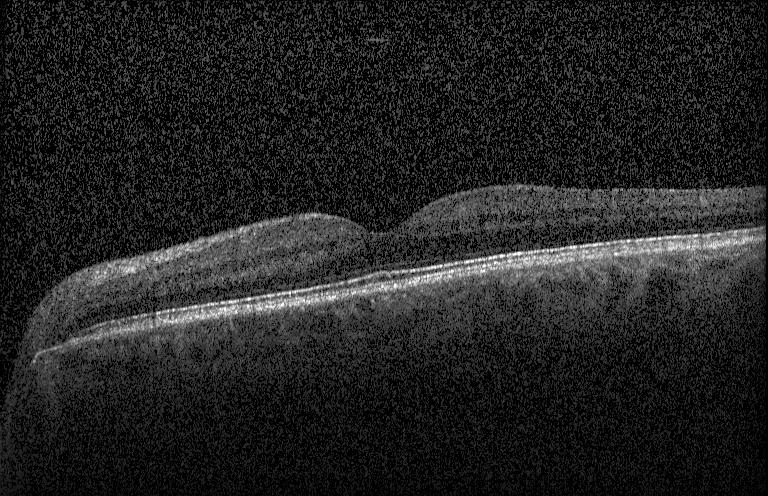 Retinal OCT B-scan. Assessment: no CNV, DME, or drusen.